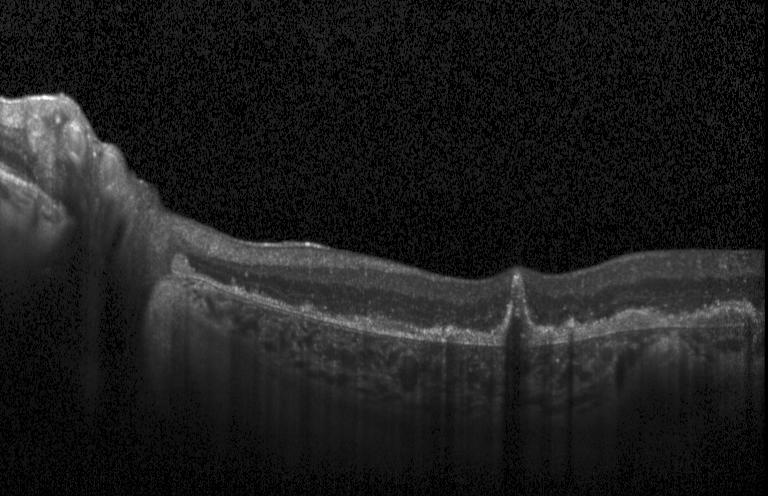
The scan shows a choroidal neovascular membrane.